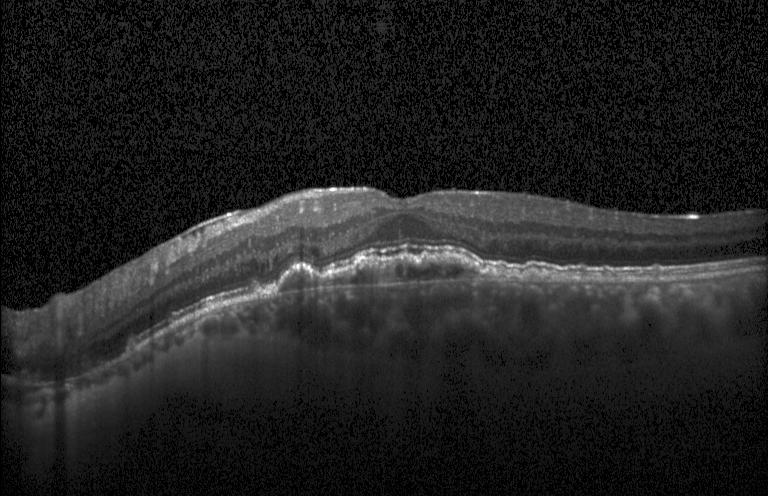
OCT finding: a choroidal neovascular membrane.